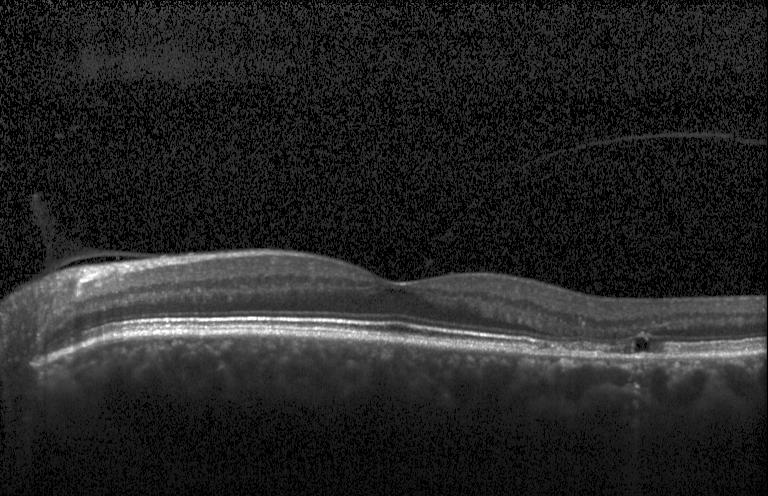
Acquired on a Heidelberg Spectralis; SD-OCT; OCT B-scan. Assessment: neither choroidal neovascularization, diabetic macular edema, nor drusen.